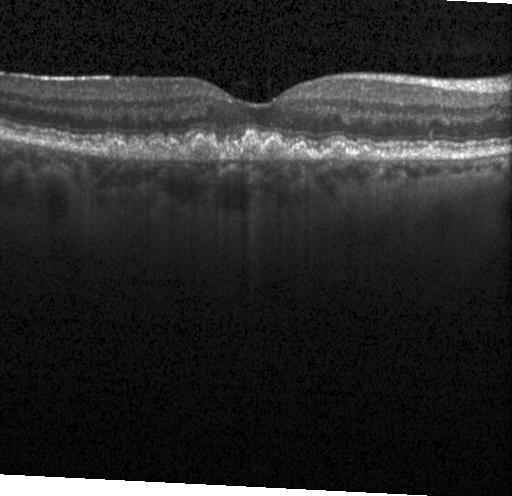

Impression: multiple drusen.